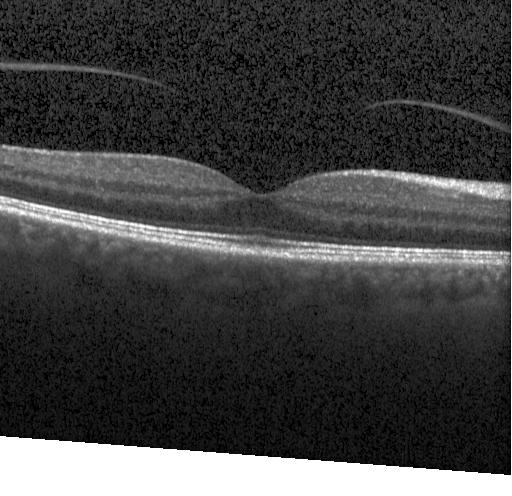 OCT B-scan, acquired on a Heidelberg Spectralis.
Finding: no evidence of CNV, DME, or drusen.